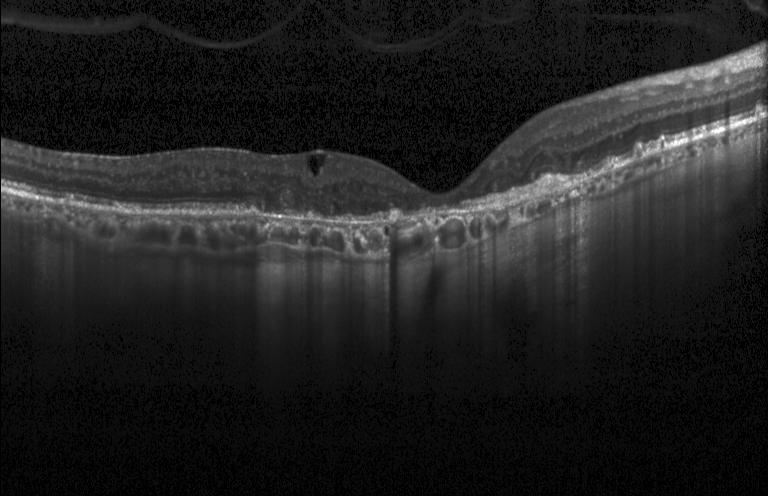 Optical coherence tomography scan · Heidelberg Spectralis OCT system · fovea-centered — Dx: a choroidal neovascular membrane.